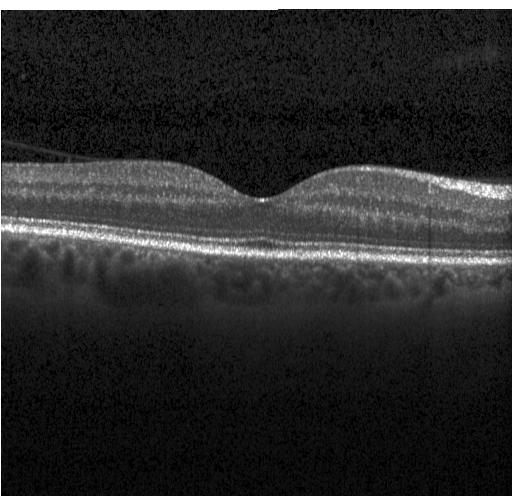 Retinal OCT B-scan.
Impression: no choroidal neovascularization, no diabetic macular edema, and no drusen.